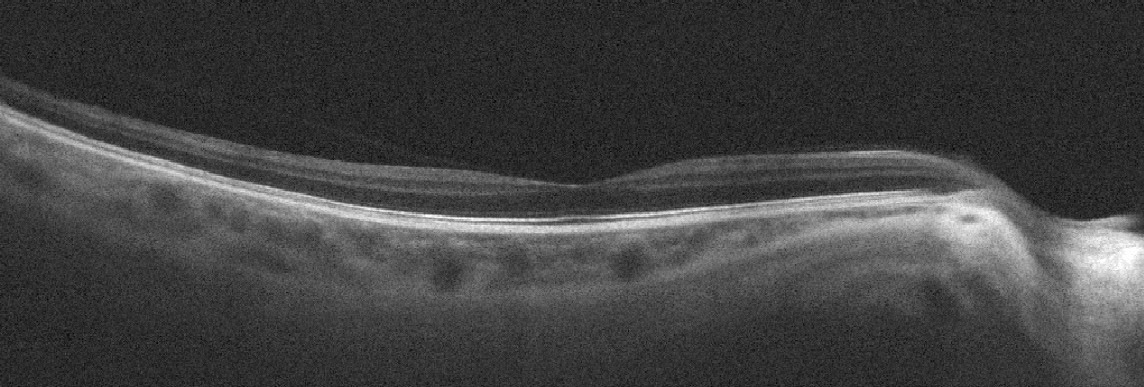
Acquired on an Optovue Avanti RTVue XR, retinal OCT cross-section
Finding: no AMD, DME, ERM, RAO, RVO, or VID.